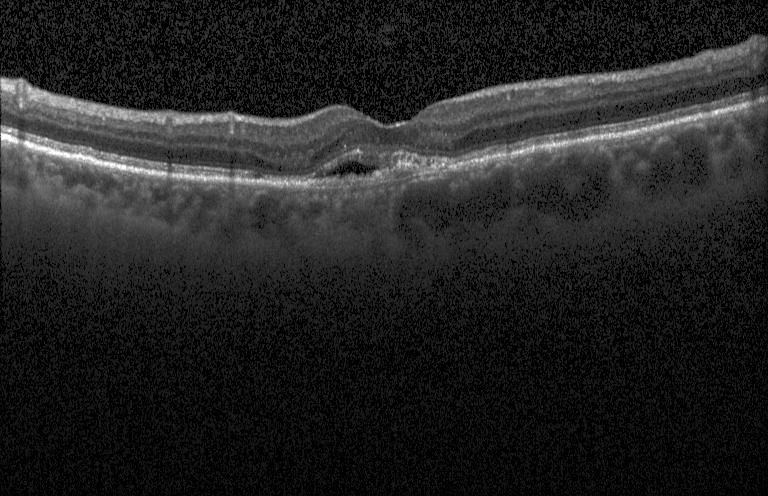 Optical coherence tomography B-scan; macular scan.
Diagnosis: a choroidal neovascular membrane.